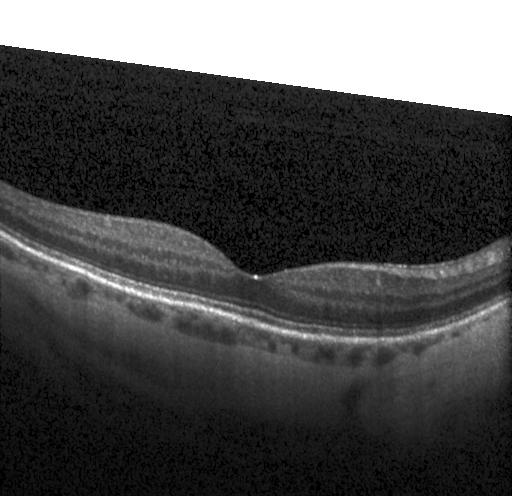 Assessment: no choroidal neovascularization, no diabetic macular edema, and no drusen.